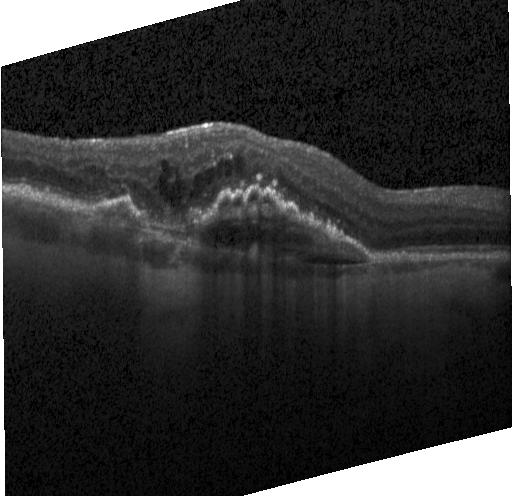

Centered on the fovea, OCT line scan
This B-scan demonstrates choroidal neovascularization (CNV).